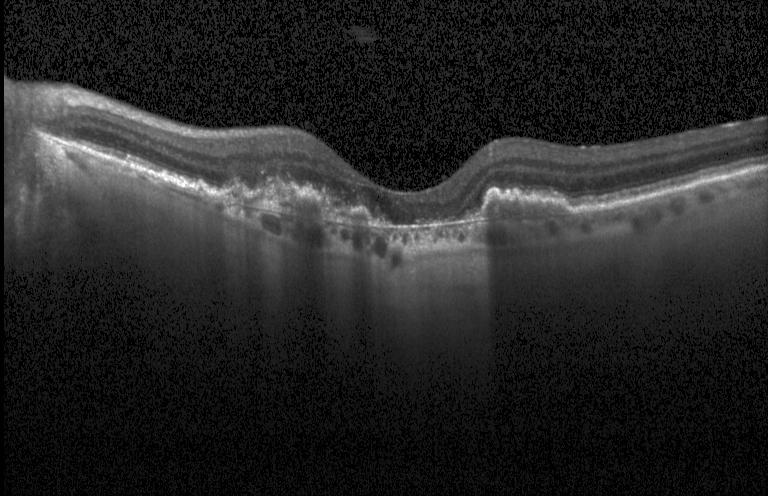

Optical coherence tomography scan. OCT finding: a choroidal neovascular membrane.